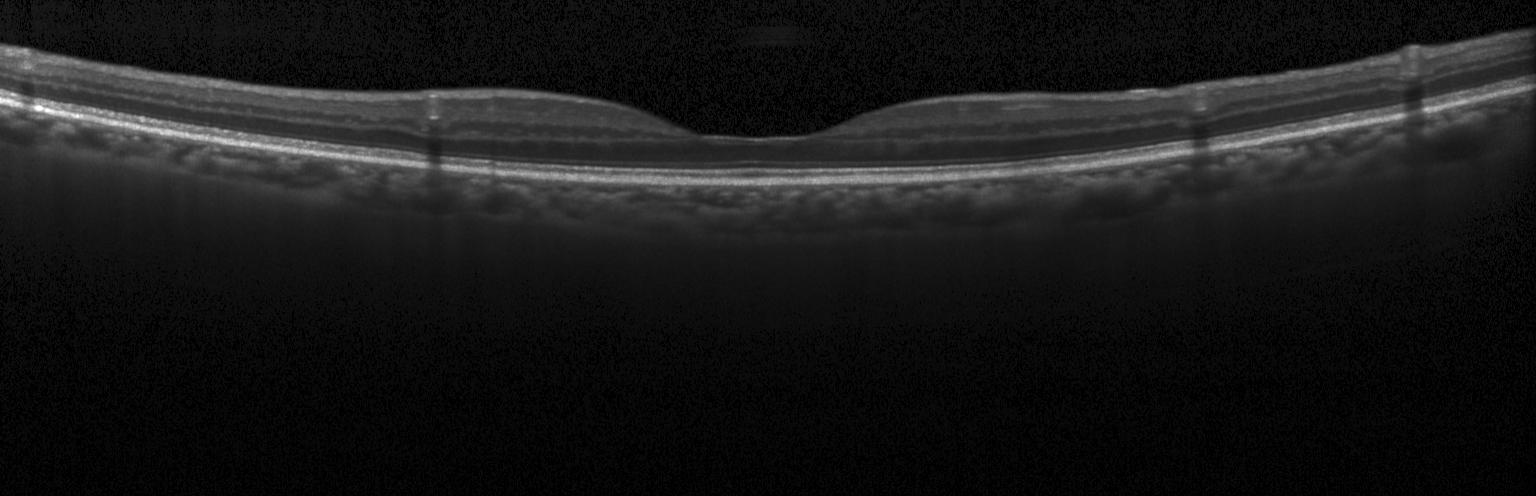 Spectral-domain OCT B-scan: no CNV, no DME, and no drusen.